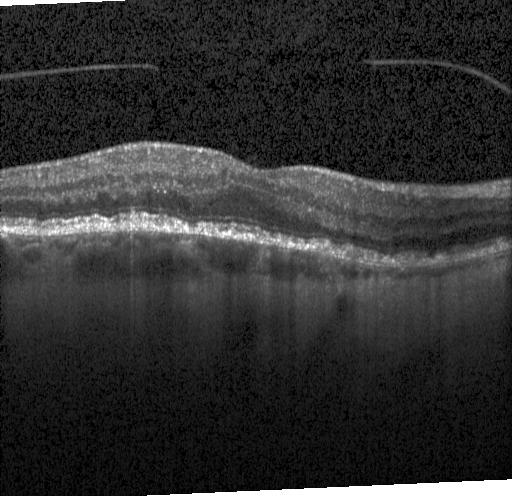
Fovea-centered, optical coherence tomography scan. Diagnosis: sub-RPE drusenoid deposits.